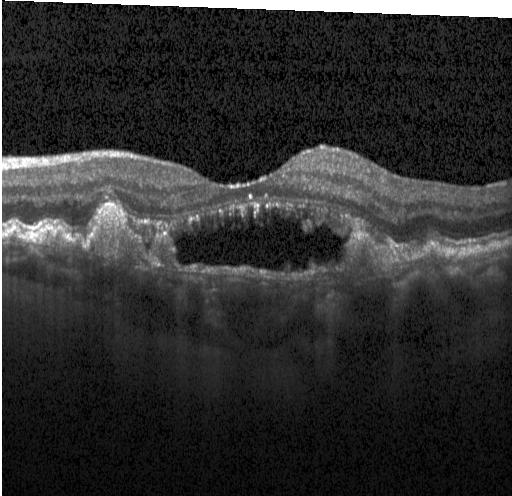

Diagnosis: CNV.